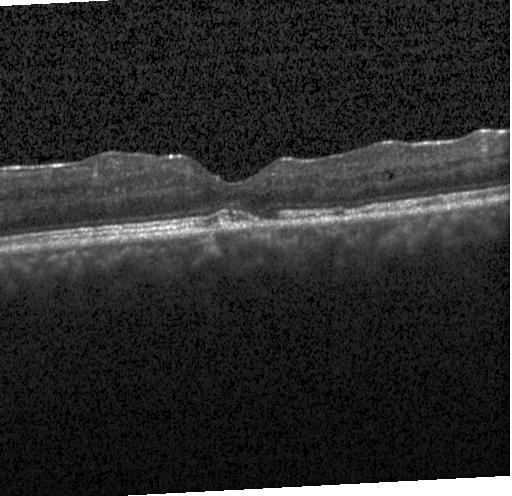
Spectral-domain OCT, fovea-centered, Heidelberg Spectralis, OCT B-scan. Multiple drusen.